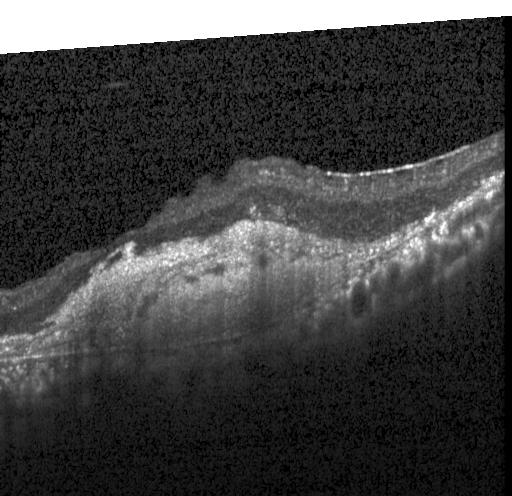 OCT scan showing CNV.